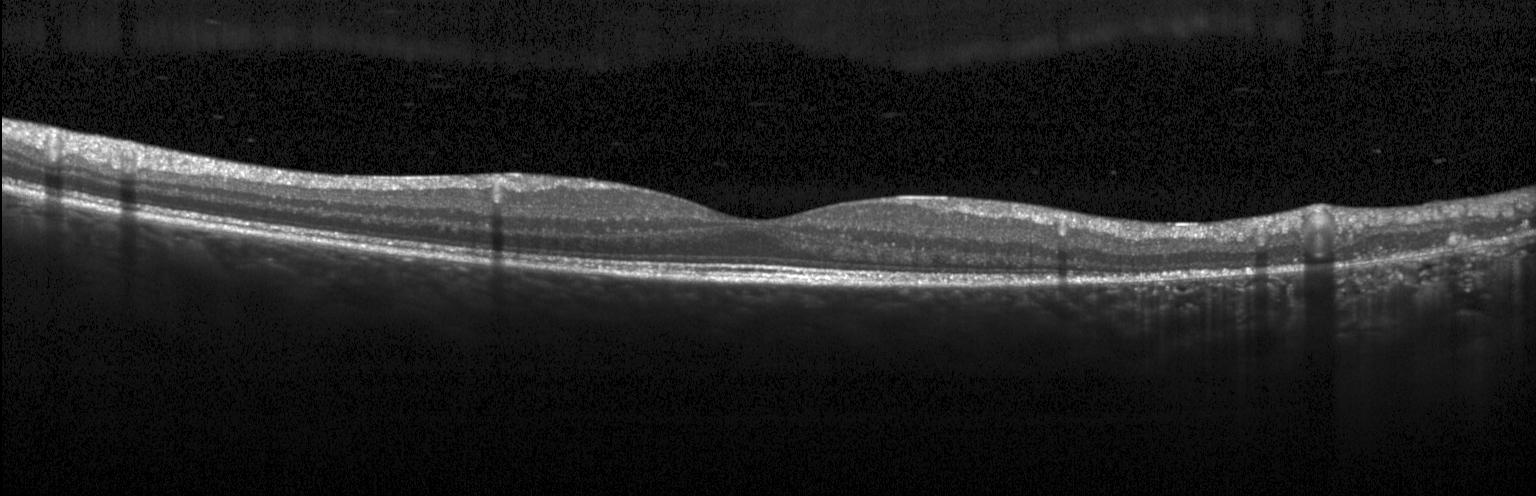
Optical coherence tomography scan, spectral-domain OCT — Dx: no evidence of CNV, DME, or drusen.